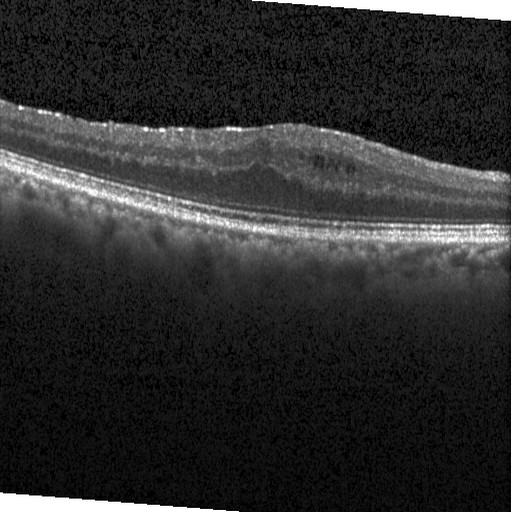
Assessment: DME.